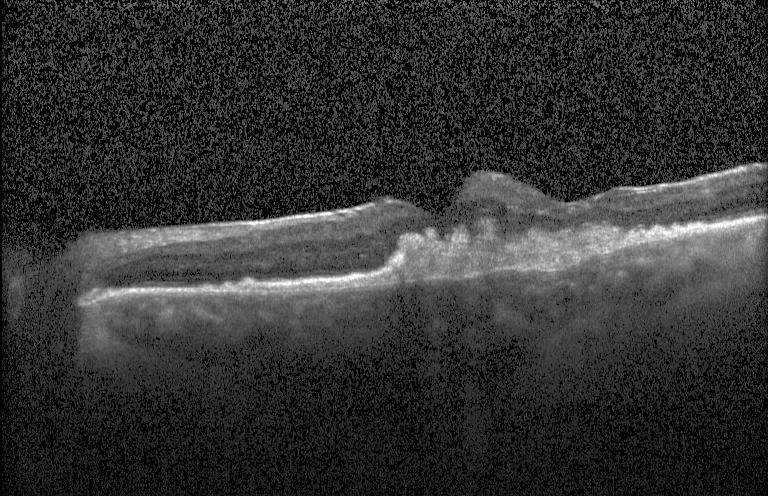
Retinal OCT B-scan. Spectral-domain optical coherence tomography
Finding: CNV.